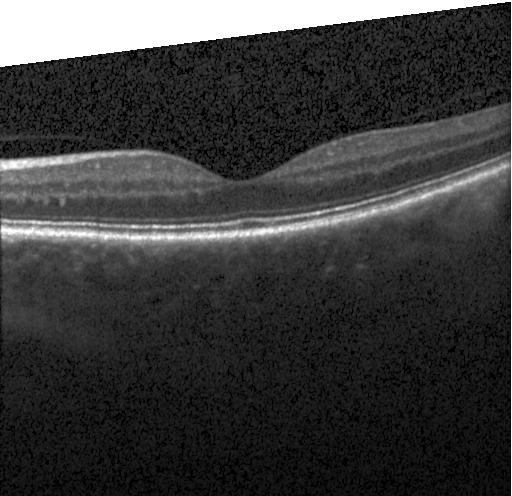
Retinal OCT cross-section. OCT finding: no choroidal neovascularization, diabetic macular edema, or drusen.